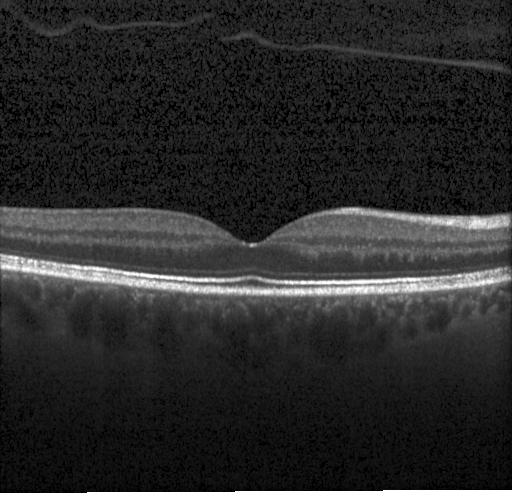 Retinal OCT cross-section. This B-scan demonstrates no evidence of choroidal neovascularization, diabetic macular edema, or drusen.